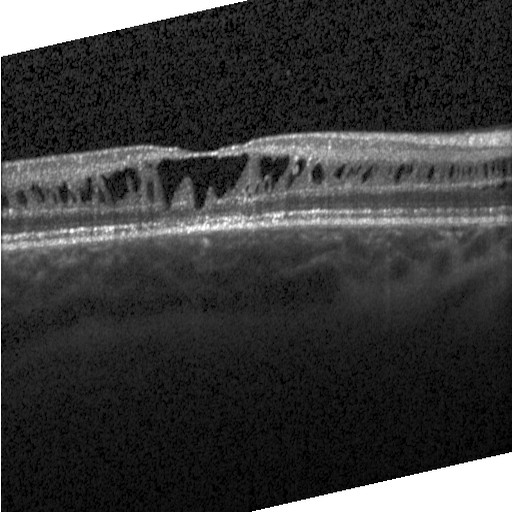
Finding: diabetic macular edema.